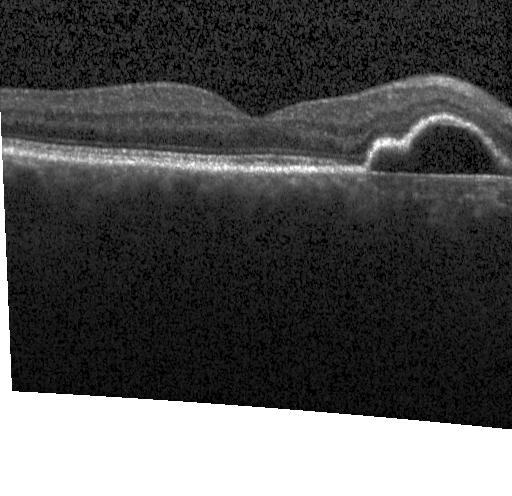 OCT finding: a choroidal neovascular membrane.